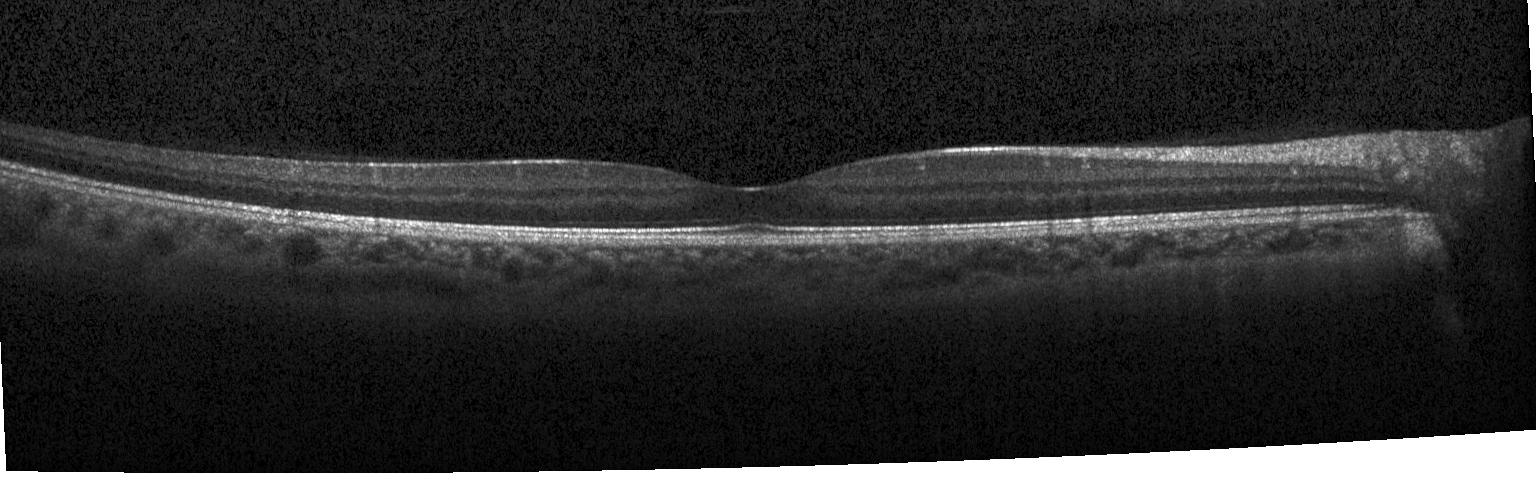

Macular OCT: no evidence of CNV, DME, or drusen.